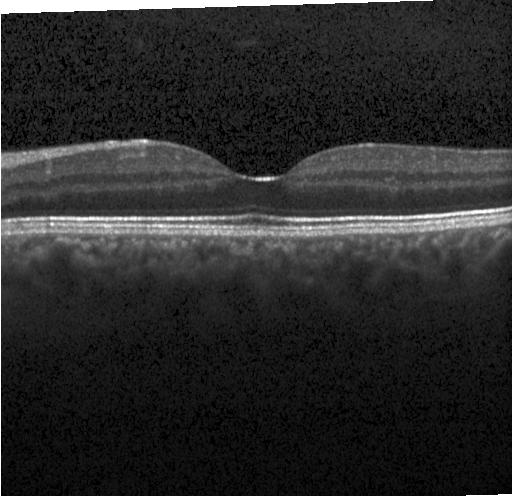

Finding: no choroidal neovascularization, diabetic macular edema, or drusen.